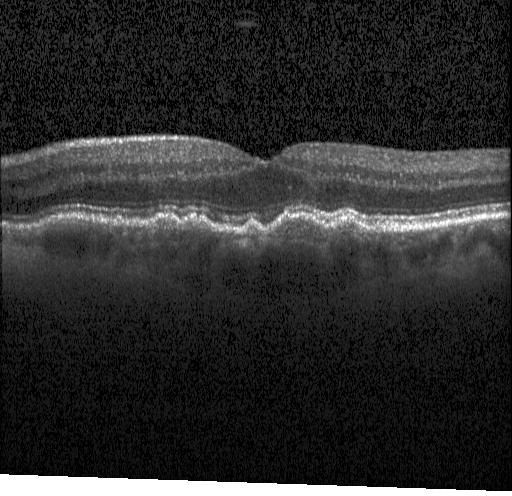

Retinal OCT cross-section showing sub-RPE drusenoid deposits.